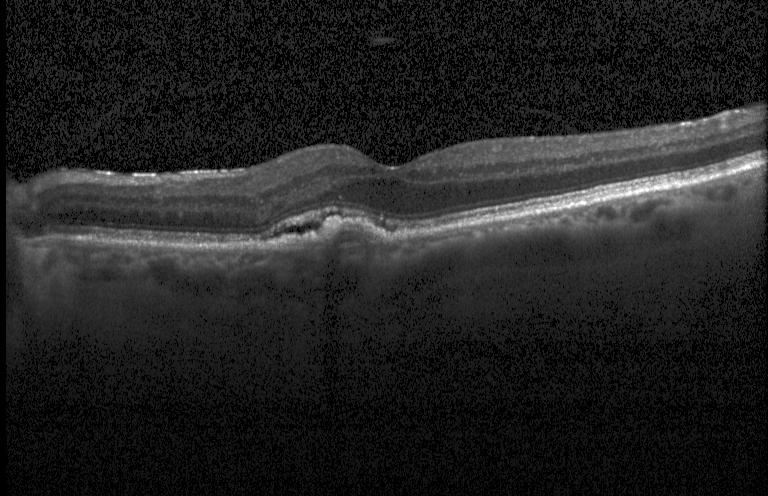
Spectral-domain optical coherence tomography, retinal OCT cross-section, centered on the fovea, Heidelberg Spectralis
Impression: a choroidal neovascular membrane.